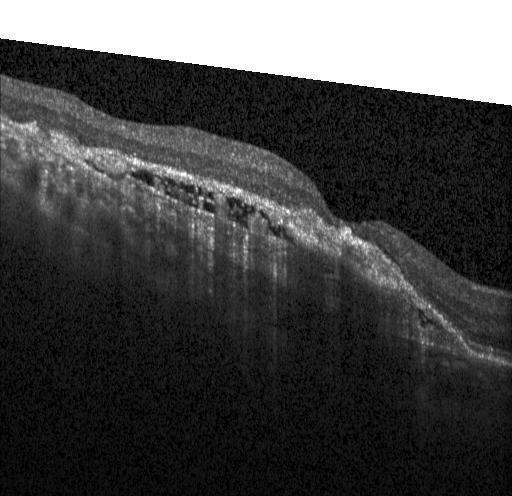 OCT B-scan · through the macula.
Macular OCT: choroidal neovascularization (CNV).